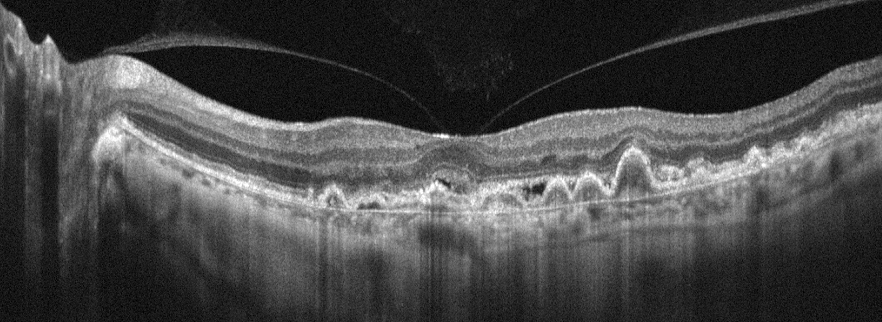

Optovue Avanti RTVue XR; macular scan; oculus sinister; OCT line scan — Finding: AMD.